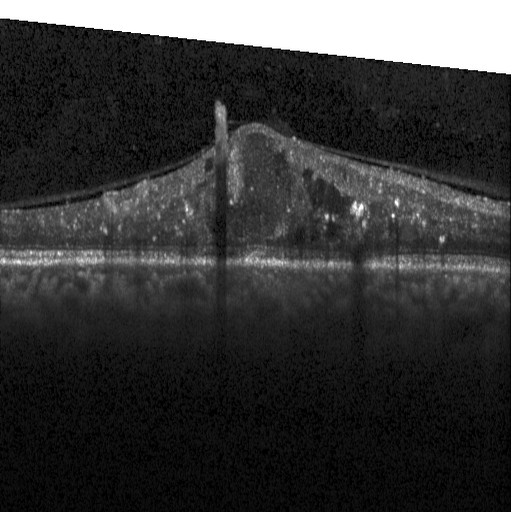
Horizontal scan through the fovea, OCT B-scan, SD-OCT. Finding: diabetic macular edema (DME).